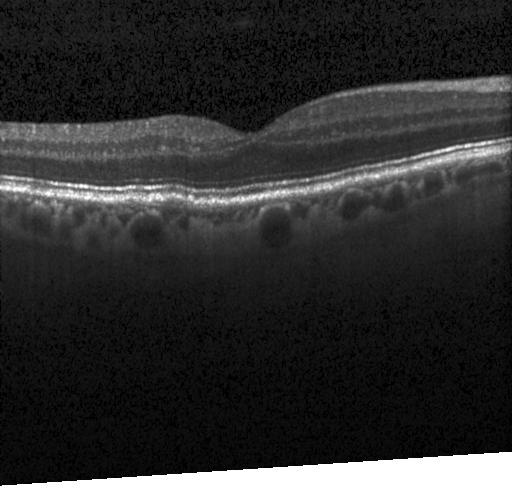

Macular scan · SD-OCT · optical coherence tomography scan
Dx: drusen.